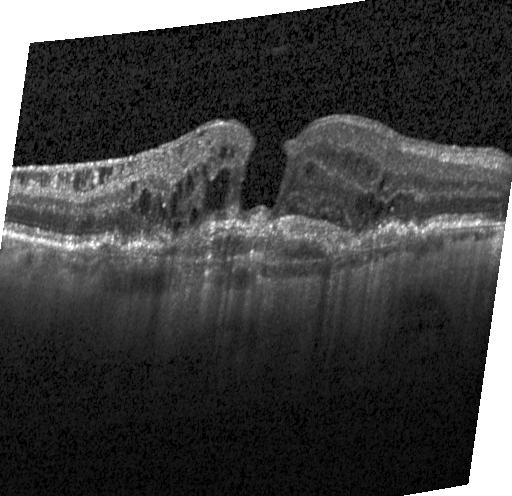 OCT B-scan — OCT finding: a choroidal neovascular membrane.